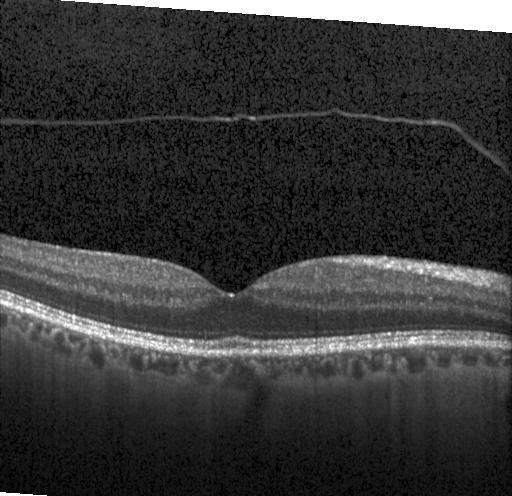

Fovea-centered; instrument: Heidelberg Spectralis; retinal OCT B-scan; SD-OCT — This B-scan demonstrates no evidence of choroidal neovascularization, diabetic macular edema, or drusen.